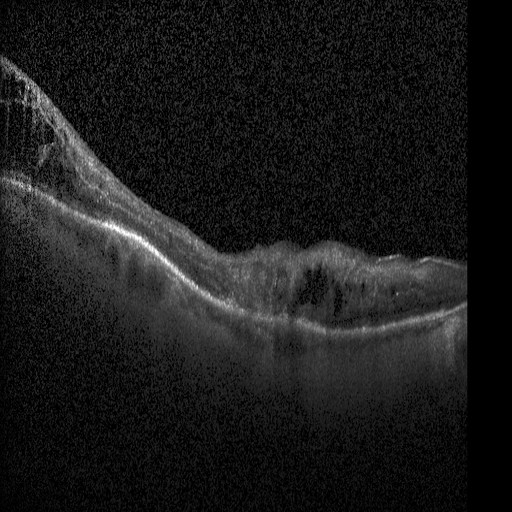
Through the macula. Spectral-domain optical coherence tomography. Heidelberg Spectralis. Retinal OCT cross-section. Dx: diabetic macular edema (DME).